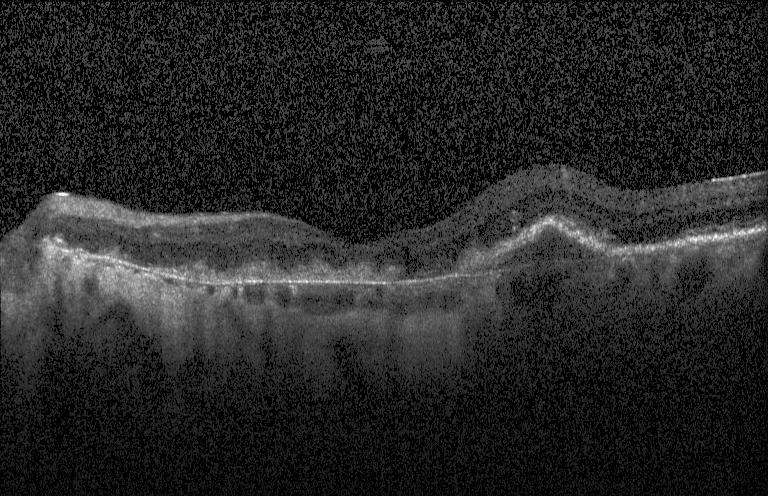
Assessment: choroidal neovascularization.